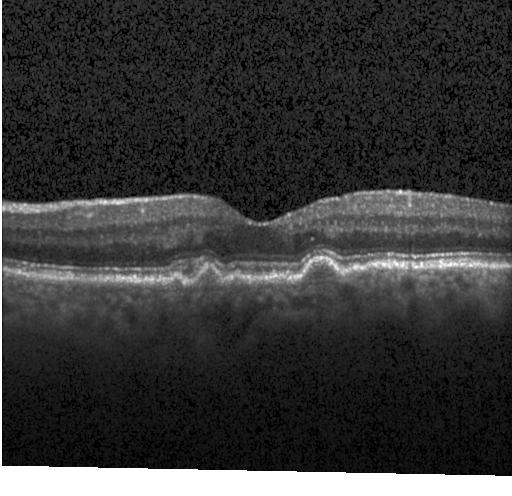
SD-OCT; OCT B-scan.
Macular OCT: multiple drusen.